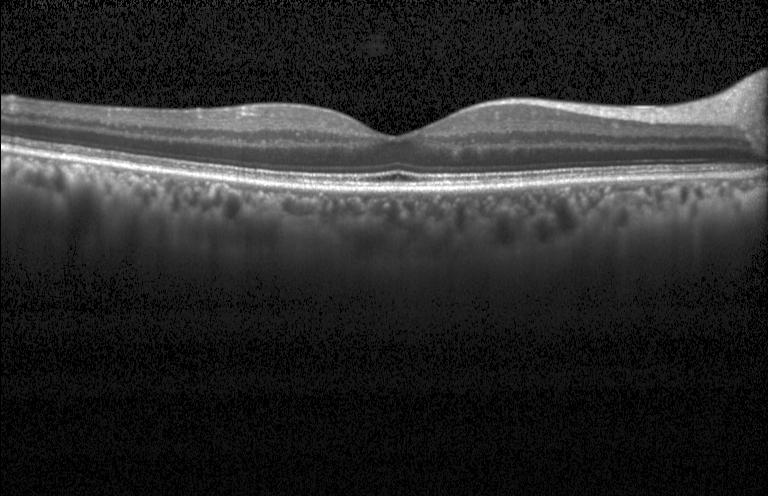
Spectral-domain OCT B-scan: neither choroidal neovascularization, diabetic macular edema, nor drusen.